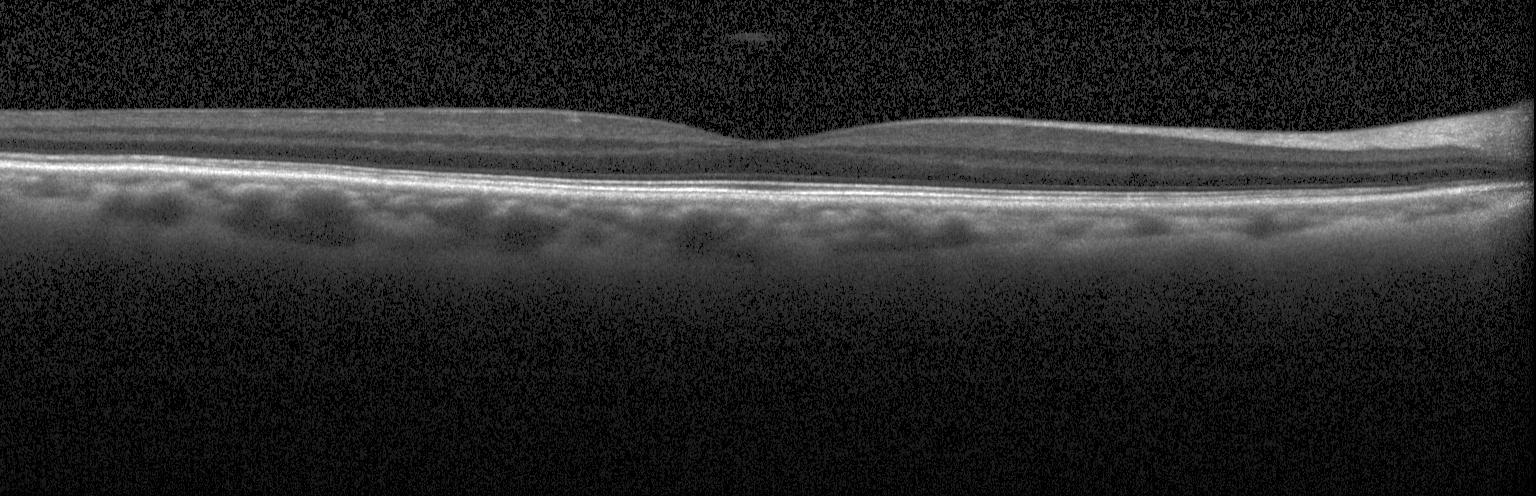

Spectral-domain OCT; centered on the fovea; optical coherence tomography scan; Heidelberg Spectralis OCT system
Impression: no evidence of choroidal neovascularization, diabetic macular edema, or drusen.